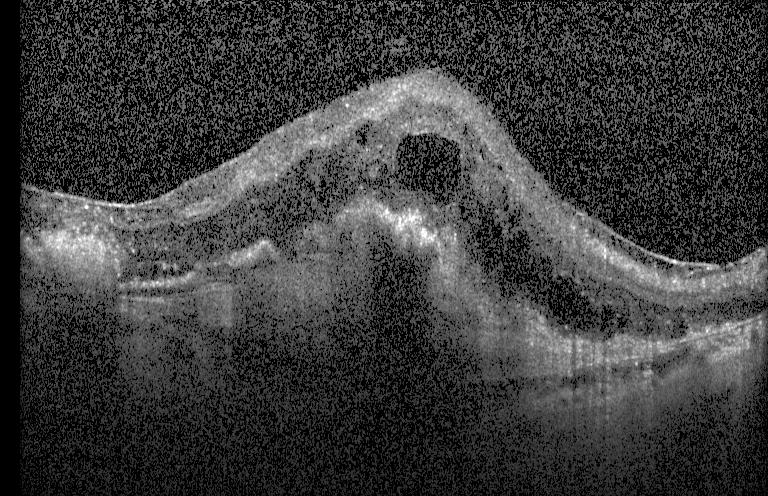 OCT B-scan.
Diagnosis: choroidal neovascularization (CNV).